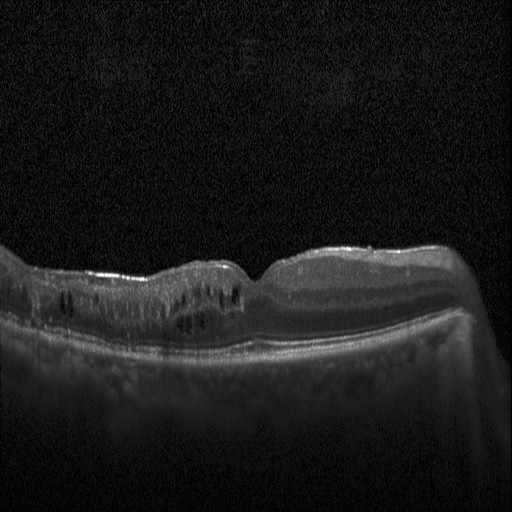
Macular scan. Optical coherence tomography B-scan. Heidelberg Spectralis OCT system
Impression: DME.